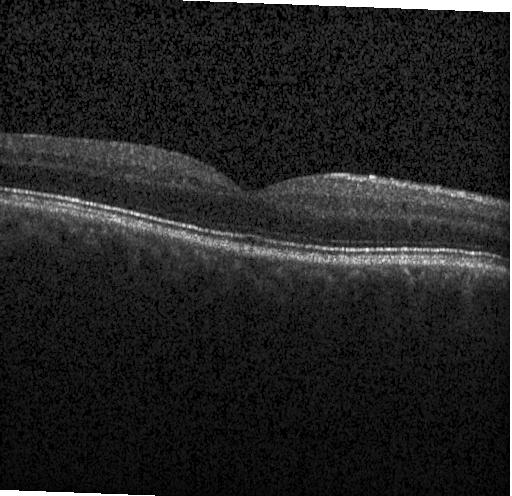
Acquired on a Heidelberg Spectralis, horizontal scan through the fovea, spectral-domain optical coherence tomography, OCT line scan.
Diagnosis: no evidence of choroidal neovascularization, diabetic macular edema, or drusen.